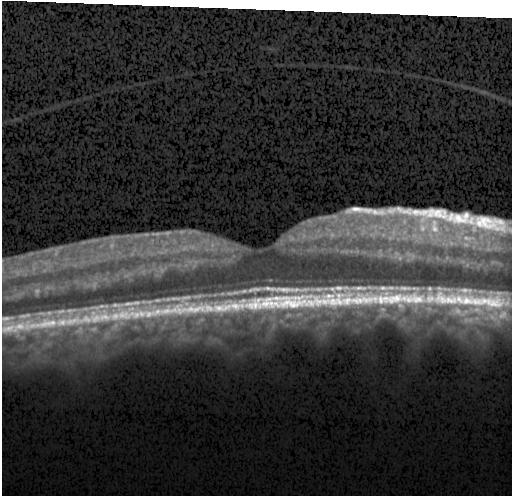
Through the macula · instrument: Heidelberg Spectralis · spectral-domain optical coherence tomography · optical coherence tomography B-scan — Dx: no CNV, DME, or drusen.